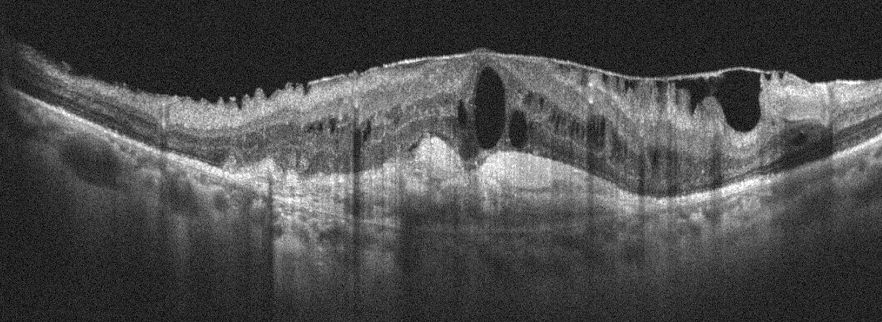

Optical coherence tomography scan · through the macula · Optovue Avanti RTVue XR — Assessment: AMD.